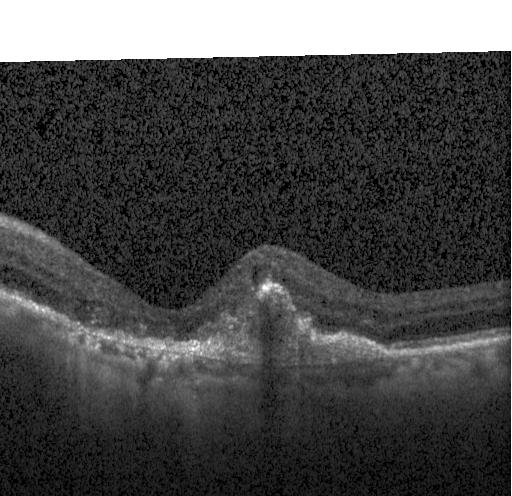

Instrument: Heidelberg Spectralis. Retinal OCT cross-section. Centered on the fovea. Spectral-domain OCT.
OCT finding: choroidal neovascularization.